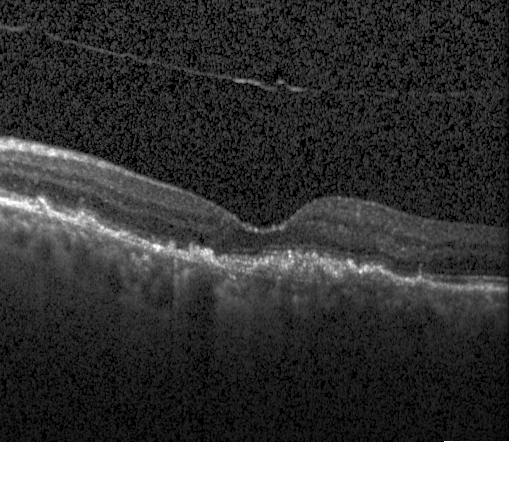 Retinal OCT cross-section showing CNV.